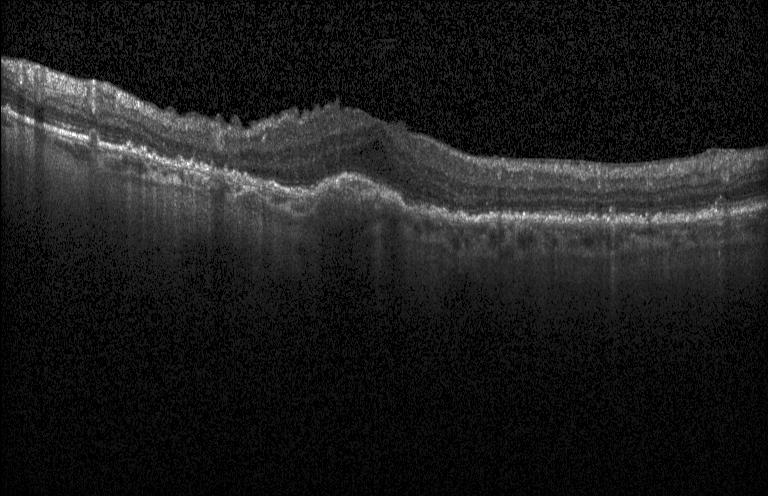

Impression: choroidal neovascularization (CNV).